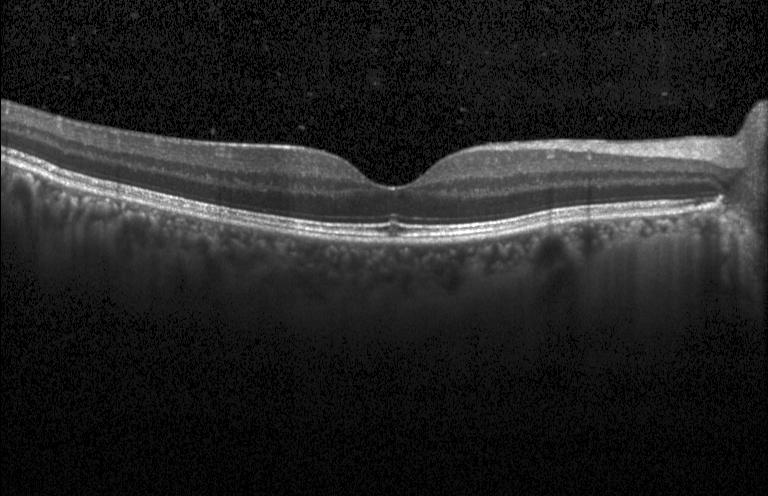
Optical coherence tomography scan — The scan shows no choroidal neovascularization, no diabetic macular edema, and no drusen.